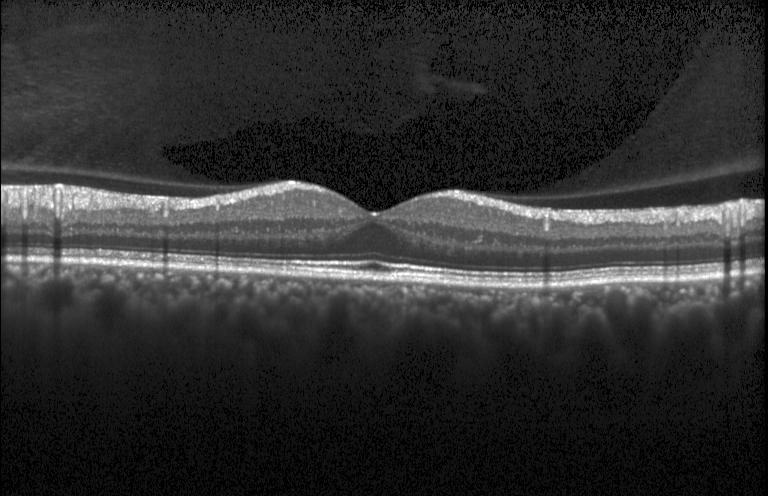
OCT scan showing no evidence of CNV, DME, or drusen.